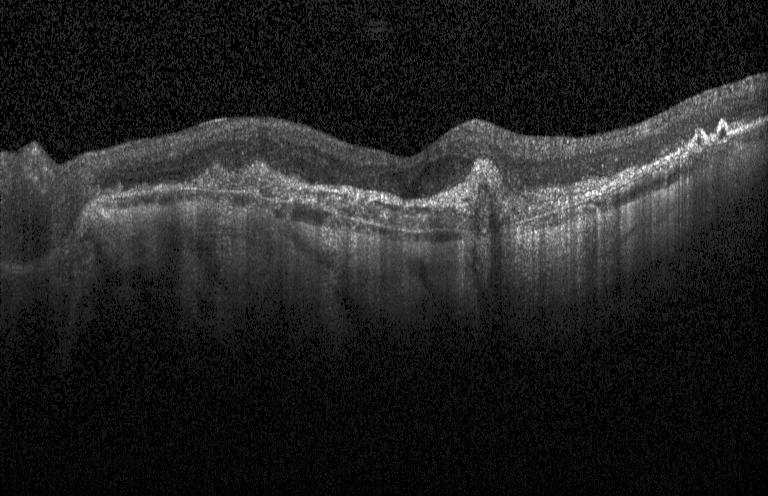

OCT B-scan · instrument: Heidelberg Spectralis. Impression: choroidal neovascularization.